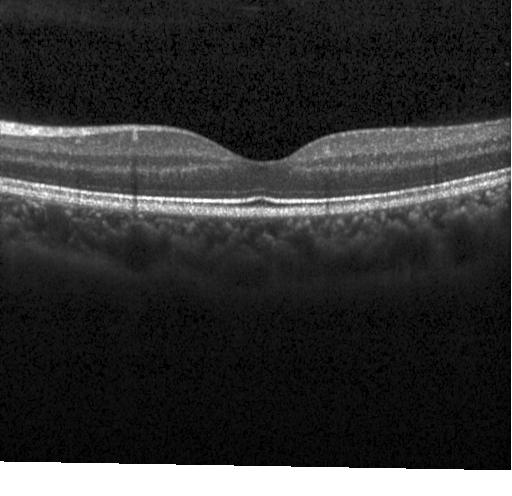
OCT scan showing no choroidal neovascularization, diabetic macular edema, or drusen.